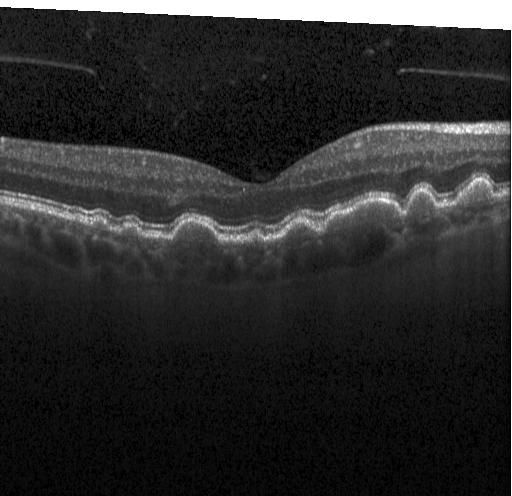 Retinal OCT B-scan. Dx: multiple drusen.